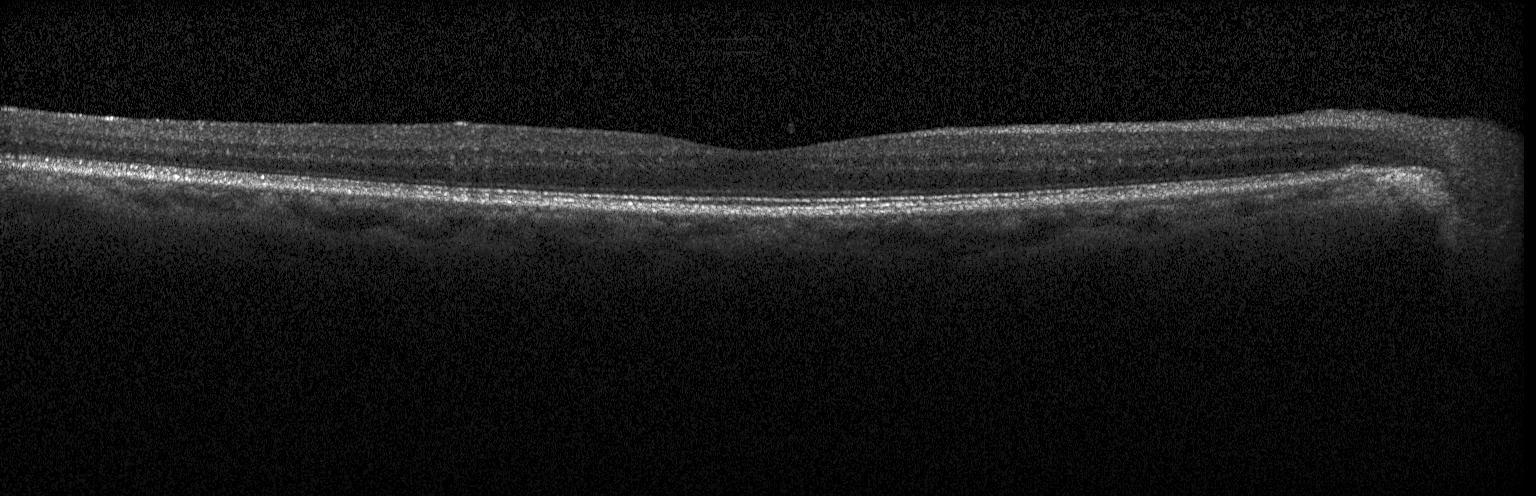

Optical coherence tomography scan.
Diagnosis: neither choroidal neovascularization, diabetic macular edema, nor drusen.